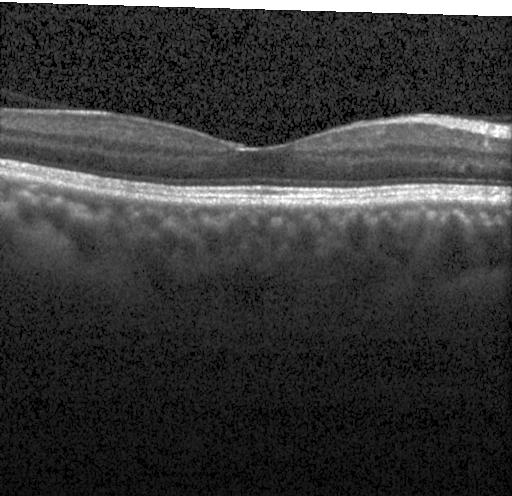 Optical coherence tomography B-scan. Dx: no evidence of choroidal neovascularization, diabetic macular edema, or drusen.